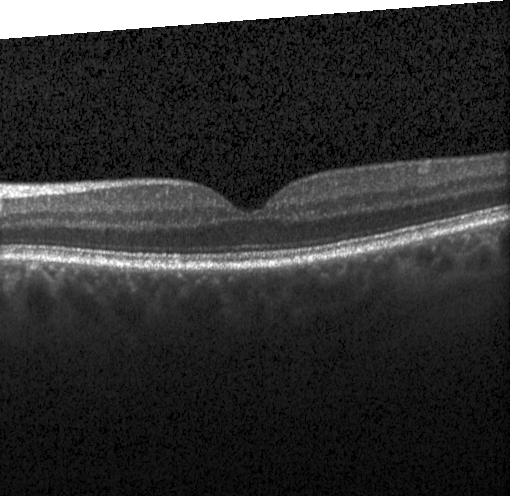
Spectral-domain OCT B-scan: no evidence of choroidal neovascularization, diabetic macular edema, or drusen.